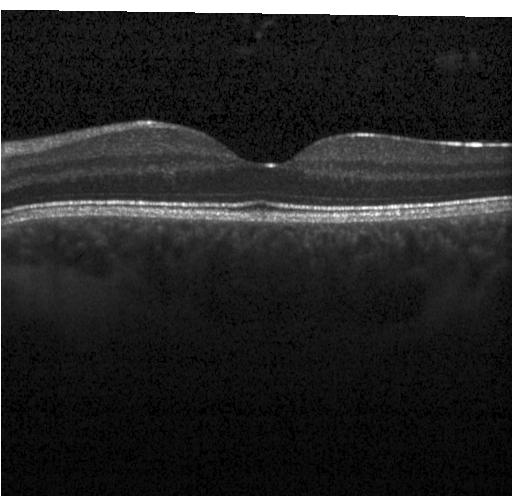
Spectral-domain OCT; retinal OCT cross-section
Impression: no choroidal neovascularization, no diabetic macular edema, and no drusen.